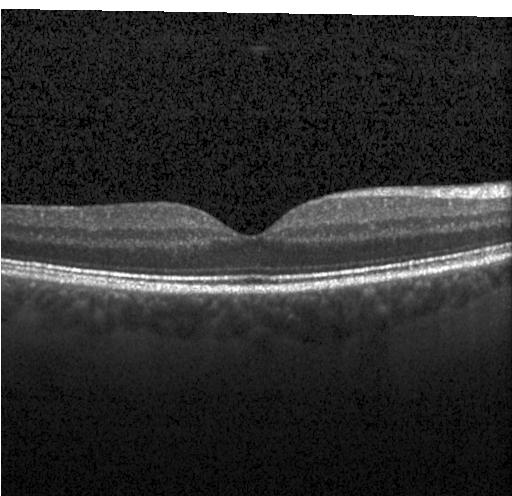
Impression: neither CNV, DME, nor drusen.